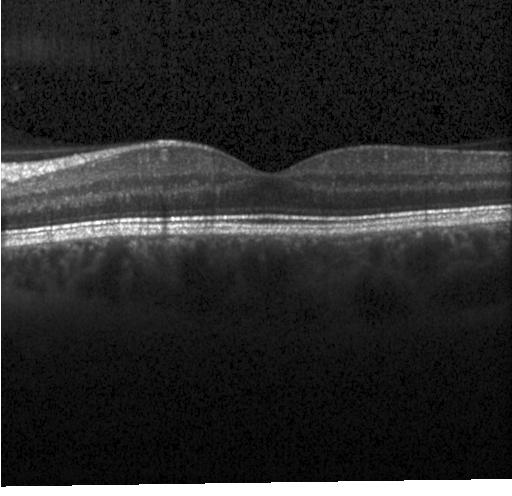 OCT B-scan; instrument: Heidelberg Spectralis; through the macula.
Impression: neither choroidal neovascularization, diabetic macular edema, nor drusen.